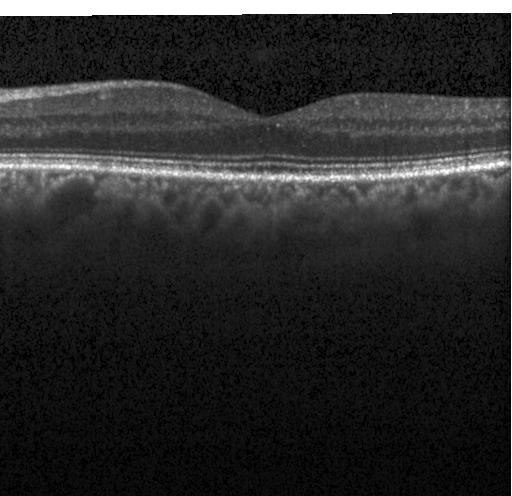 Optical coherence tomography scan, spectral-domain OCT. Impression: no CNV, no DME, and no drusen.